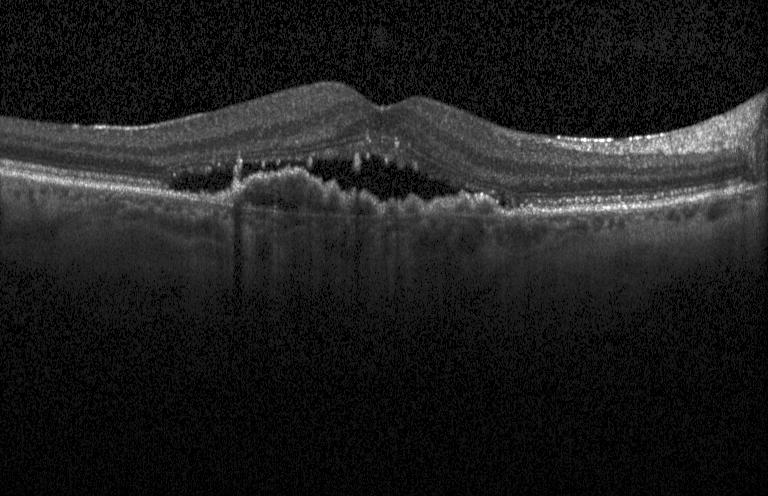

Spectral-domain OCT B-scan: CNV.